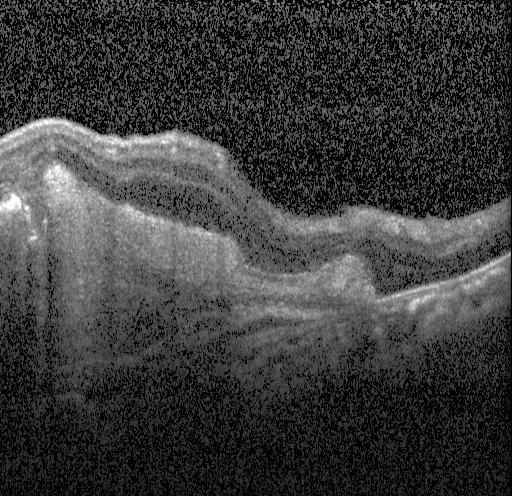
OCT B-scan — Macular OCT: CNV.